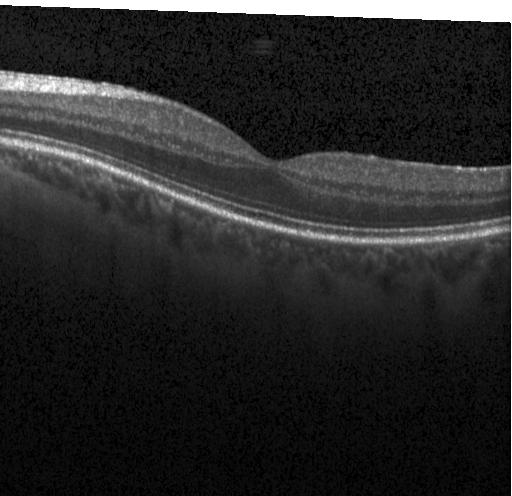
SD-OCT. Through the macula. OCT B-scan. Heidelberg Spectralis. No choroidal neovascularization, diabetic macular edema, or drusen.